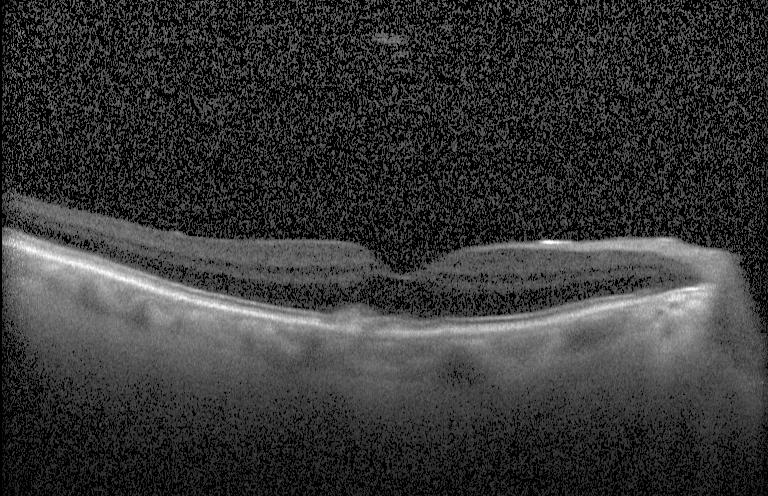 Optical coherence tomography scan. Assessment: choroidal neovascularization (CNV).